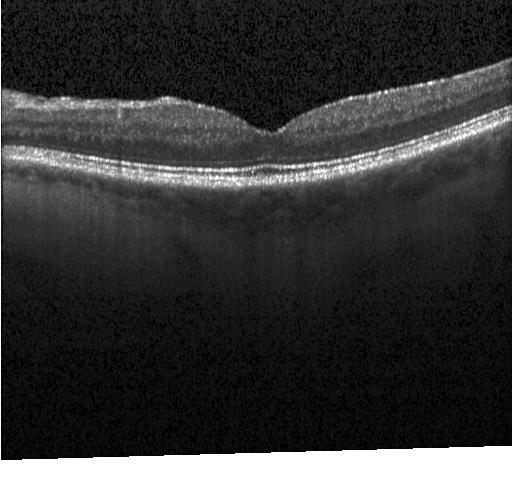

OCT line scan
Assessment: no evidence of CNV, DME, or drusen.